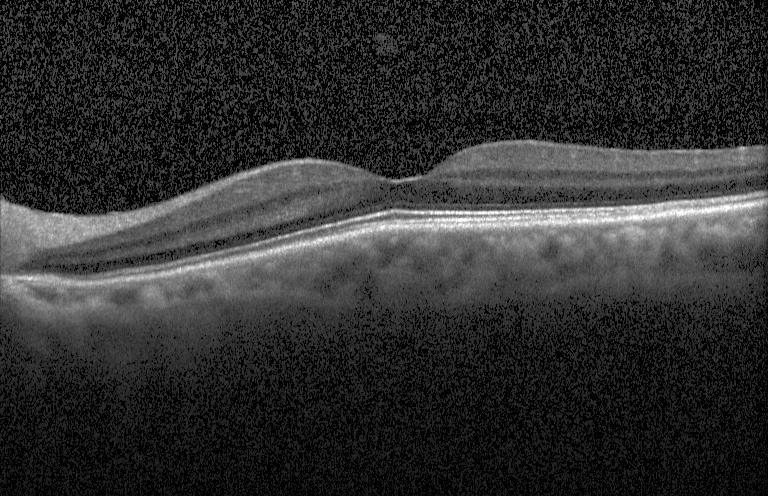
Retinal OCT cross-section, through the macula, Heidelberg Spectralis. Diagnosis: no choroidal neovascularization, no diabetic macular edema, and no drusen.